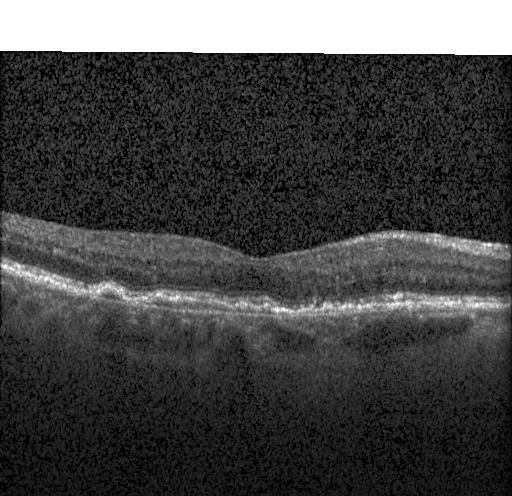
Optical coherence tomography B-scan
Diagnosis: CNV.